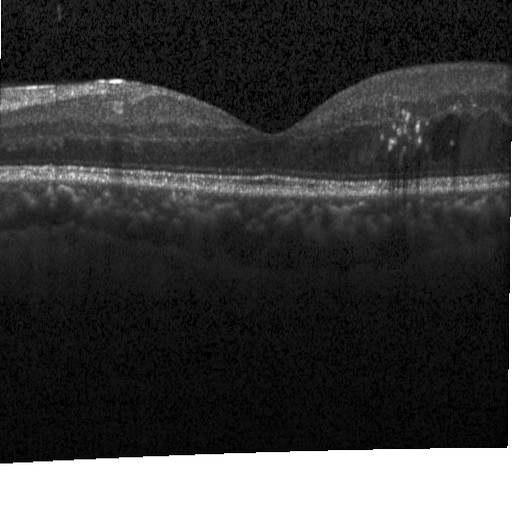

Spectral-domain optical coherence tomography; OCT B-scan — Assessment: diabetic macular edema (DME).